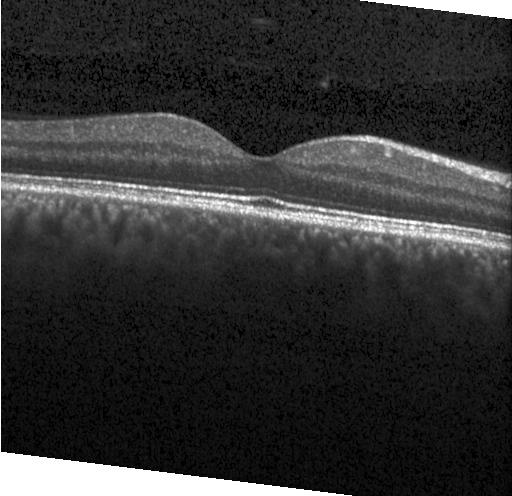
OCT B-scan showing no evidence of choroidal neovascularization, diabetic macular edema, or drusen.